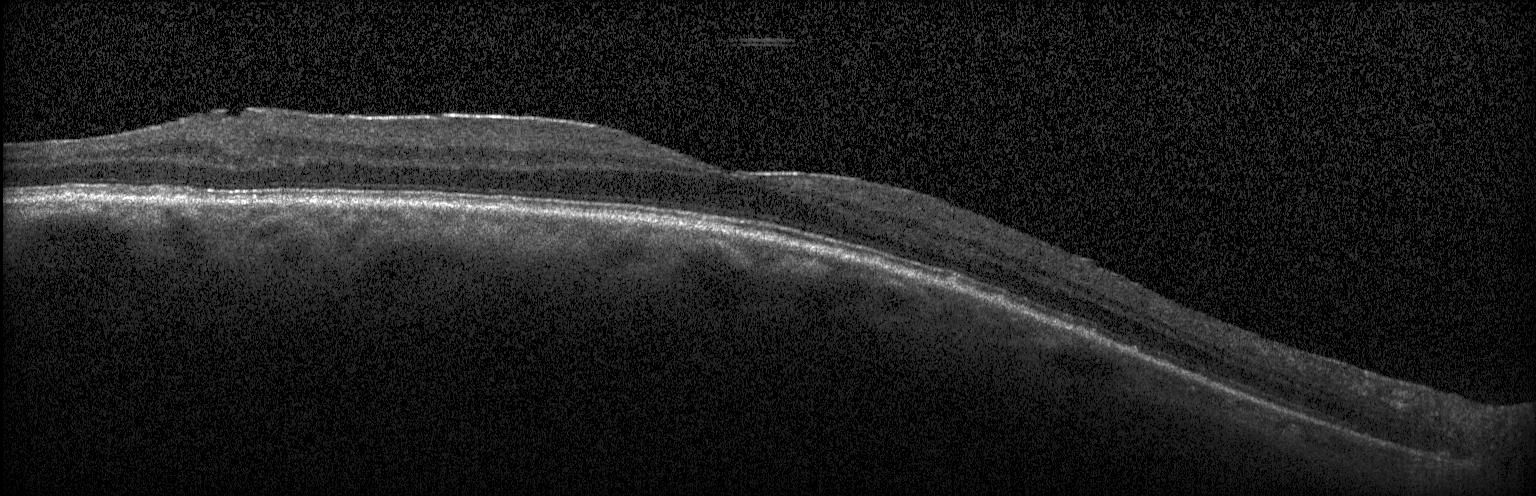 Through the macula · retinal OCT cross-section · Heidelberg Spectralis OCT system · spectral-domain optical coherence tomography — OCT finding: neither choroidal neovascularization, diabetic macular edema, nor drusen.